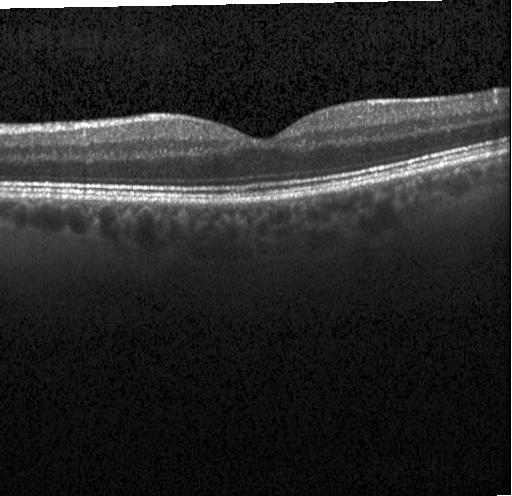 The scan shows no choroidal neovascularization, no diabetic macular edema, and no drusen.